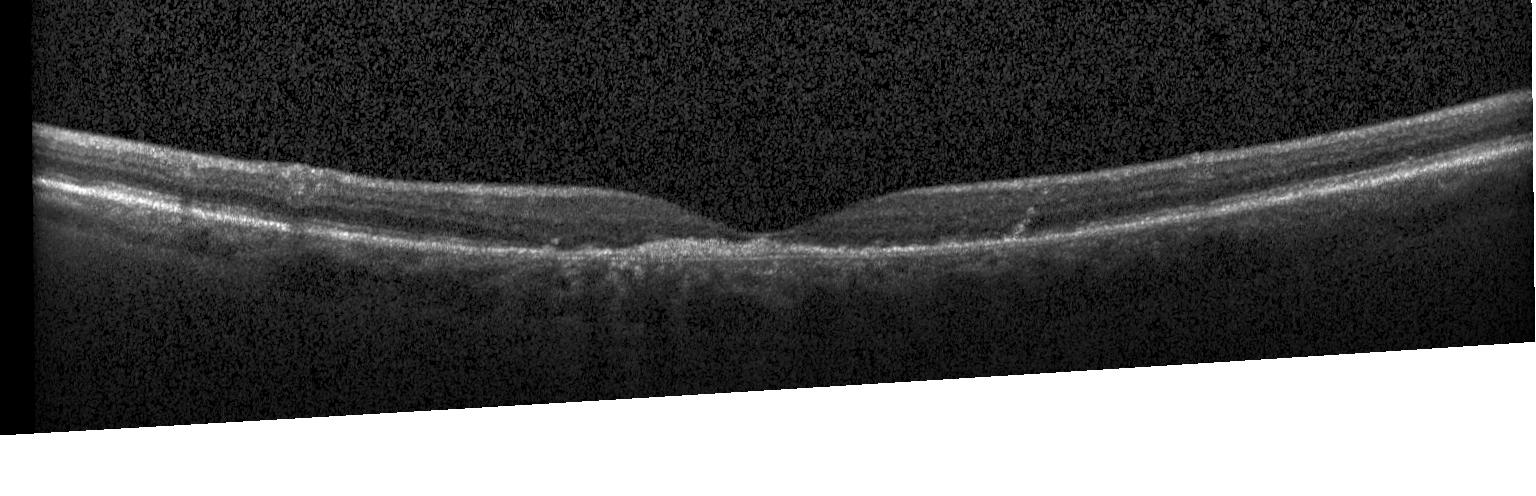
Optical coherence tomography B-scan.
Dx: choroidal neovascularization (CNV).